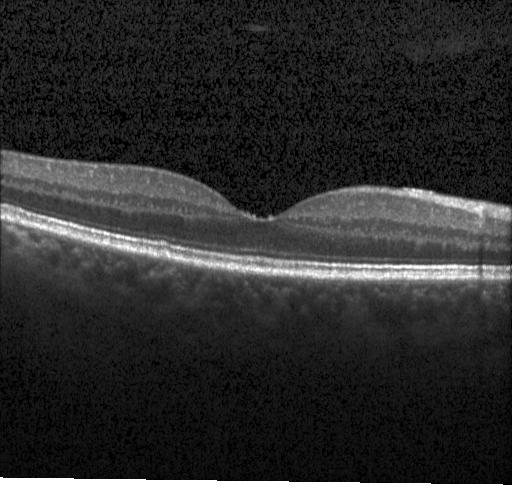 Retinal OCT cross-section showing neither CNV, DME, nor drusen.